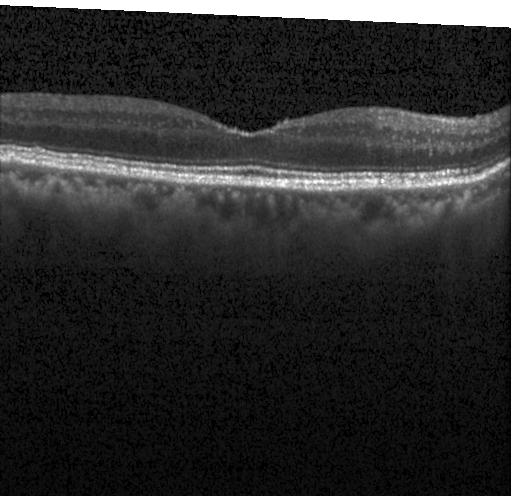
Spectral-domain optical coherence tomography, retinal OCT cross-section. This B-scan demonstrates no evidence of CNV, DME, or drusen.